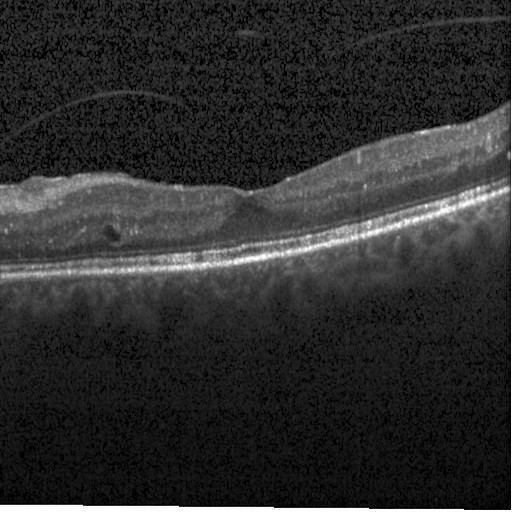 Macular OCT: DME.